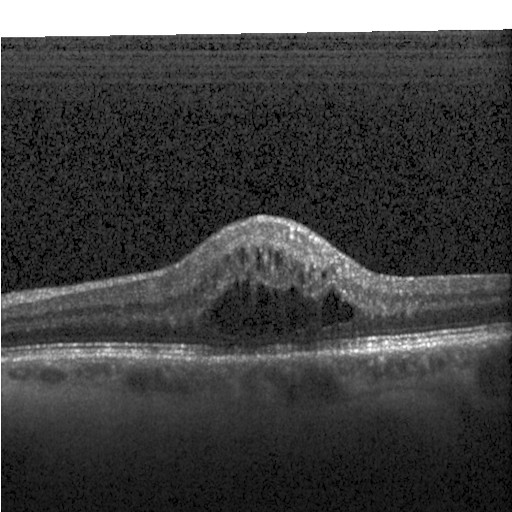
Retinal OCT cross-section. Horizontal scan through the fovea. Instrument: Heidelberg Spectralis. Spectral-domain OCT
Finding: diabetic macular edema.